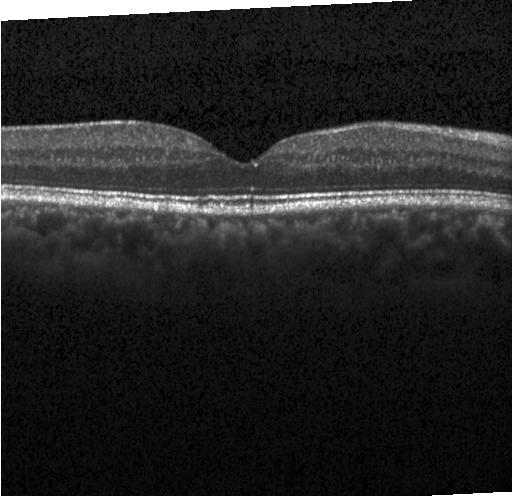

Spectral-domain optical coherence tomography; optical coherence tomography B-scan. This B-scan demonstrates no choroidal neovascularization, diabetic macular edema, or drusen.